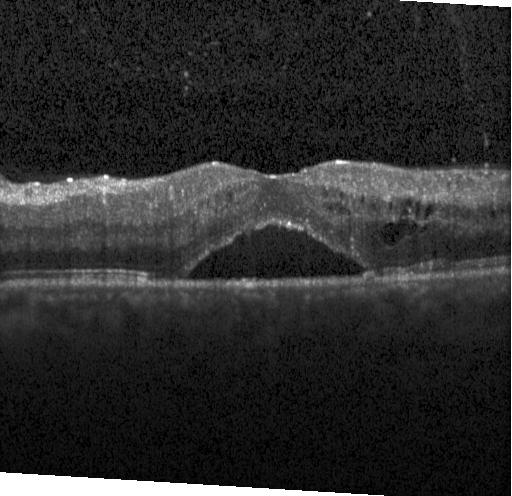
Heidelberg Spectralis OCT system · spectral-domain optical coherence tomography · OCT line scan
Diabetic macular edema (DME).